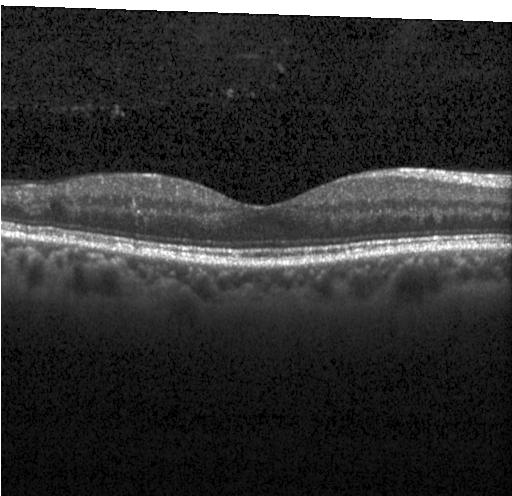
Instrument: Heidelberg Spectralis · optical coherence tomography B-scan.
Diagnosis: neither choroidal neovascularization, diabetic macular edema, nor drusen.